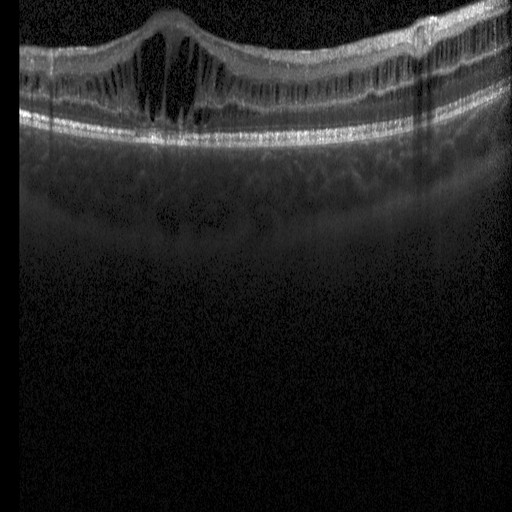 Macular scan; spectral-domain optical coherence tomography; retinal OCT B-scan; Heidelberg Spectralis OCT system
Impression: DME.